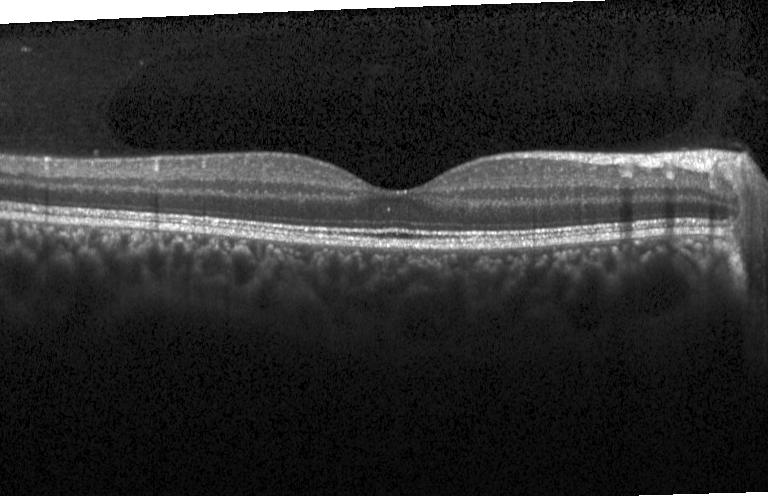 Through the macula, optical coherence tomography scan, spectral-domain OCT. OCT finding: no CNV, DME, or drusen.